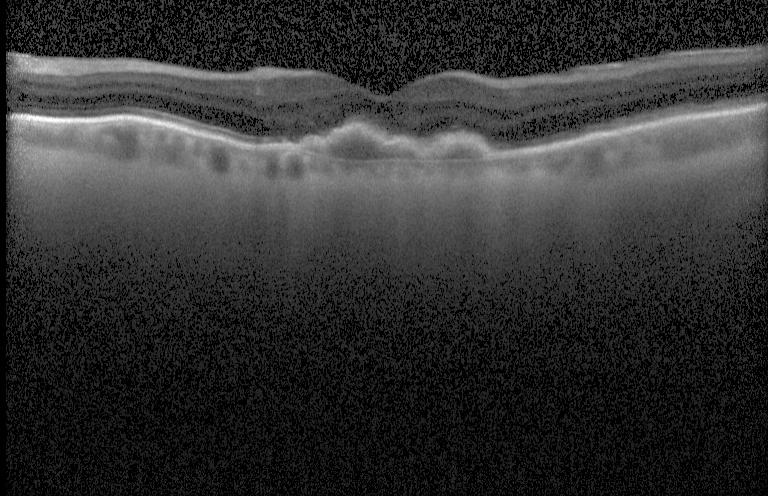

Spectral-domain OCT. Optical coherence tomography B-scan — Diagnosis: a choroidal neovascular membrane.